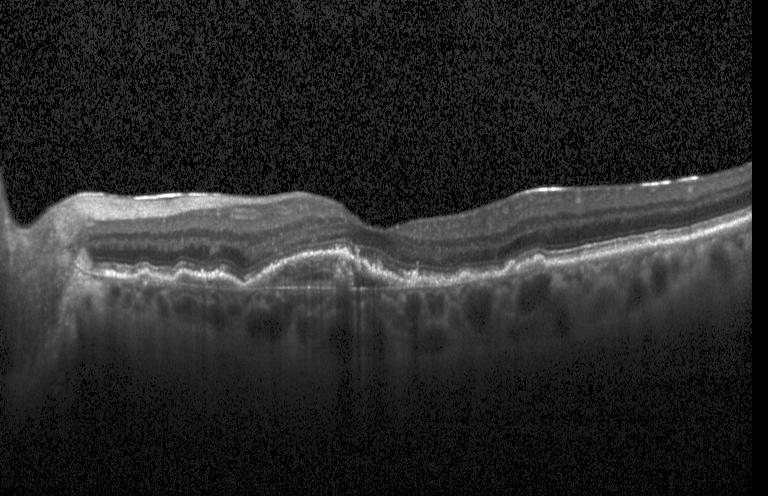

Finding: CNV.